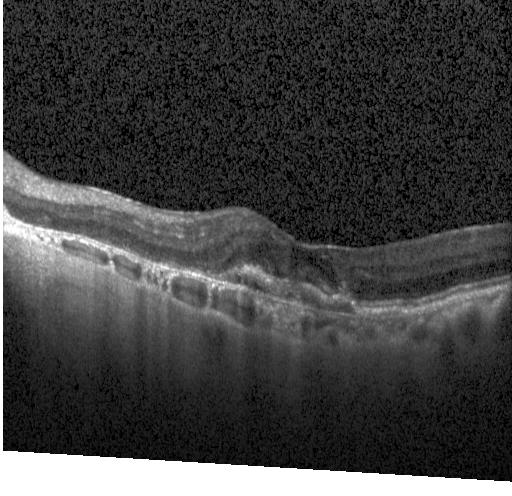 Retinal OCT cross-section; acquired on a Heidelberg Spectralis; spectral-domain optical coherence tomography
Impression: a choroidal neovascular membrane.